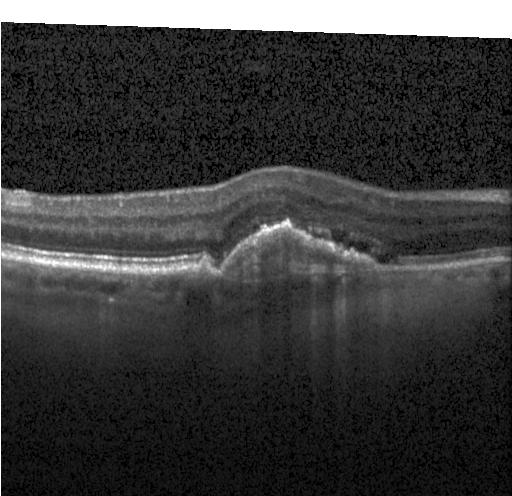

Optical coherence tomography scan, Heidelberg Spectralis — OCT finding: CNV.